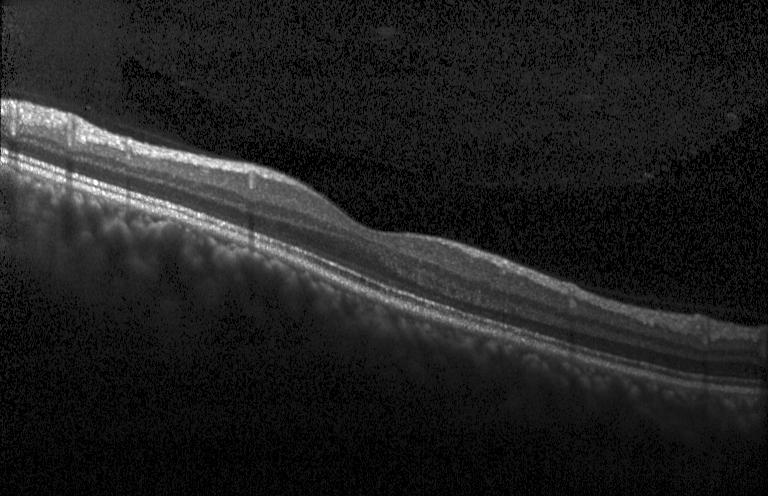 Retinal OCT B-scan. Assessment: no choroidal neovascularization, diabetic macular edema, or drusen.